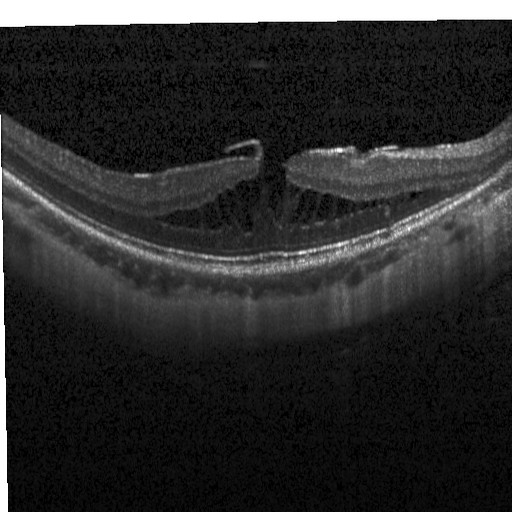
Optical coherence tomography B-scan · Heidelberg Spectralis · horizontal scan through the fovea — OCT finding: diabetic macular edema (DME).